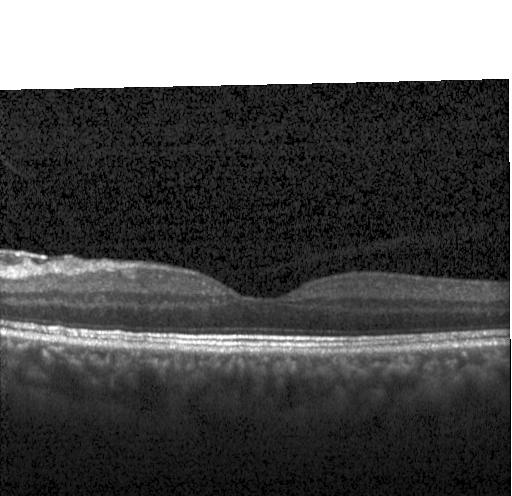 Impression: no choroidal neovascularization, no diabetic macular edema, and no drusen.